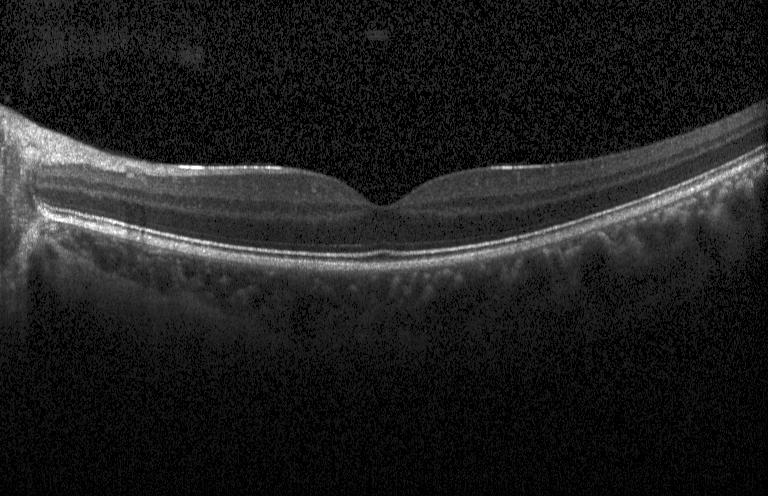
Optical coherence tomography B-scan — Finding: neither choroidal neovascularization, diabetic macular edema, nor drusen.